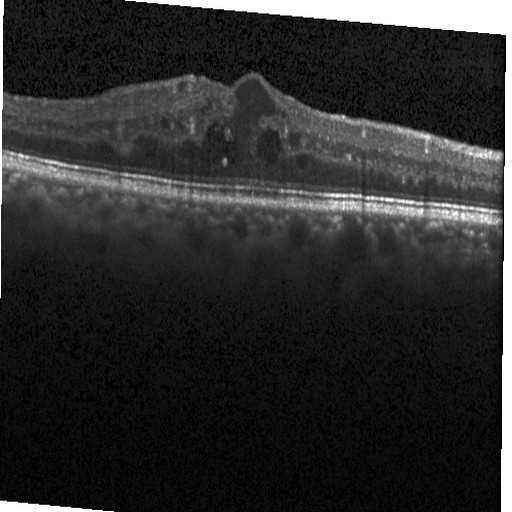

Fovea-centered. OCT line scan. Finding: diabetic macular edema (DME).